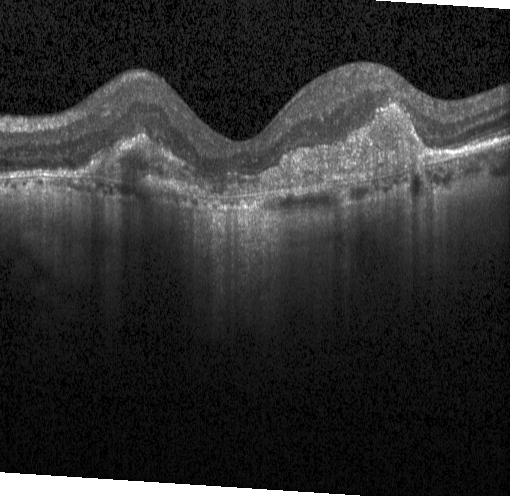 Heidelberg Spectralis OCT system · horizontal scan through the fovea · retinal OCT B-scan · spectral-domain optical coherence tomography. A choroidal neovascular membrane.